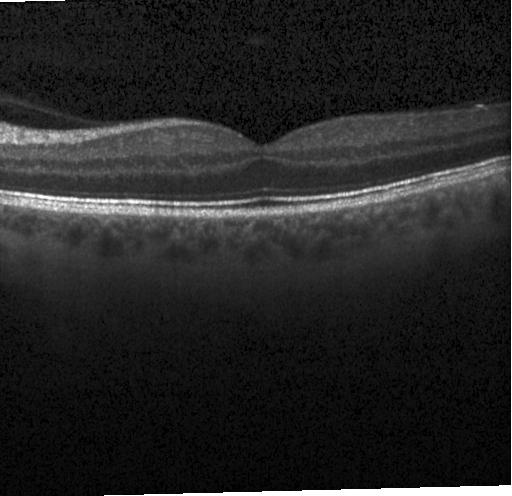 OCT scan showing neither CNV, DME, nor drusen.